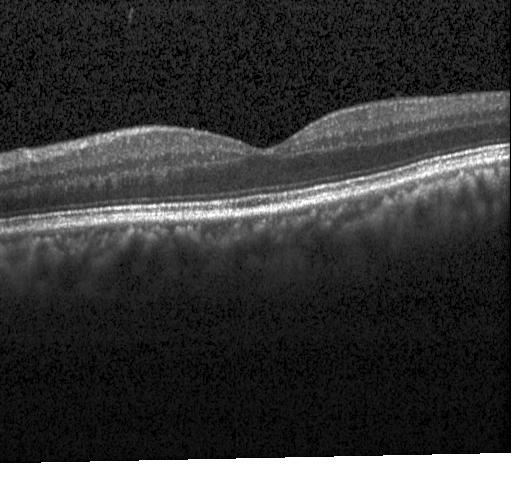 Macular scan; OCT B-scan; SD-OCT; Heidelberg Spectralis — Impression: no choroidal neovascularization, no diabetic macular edema, and no drusen.